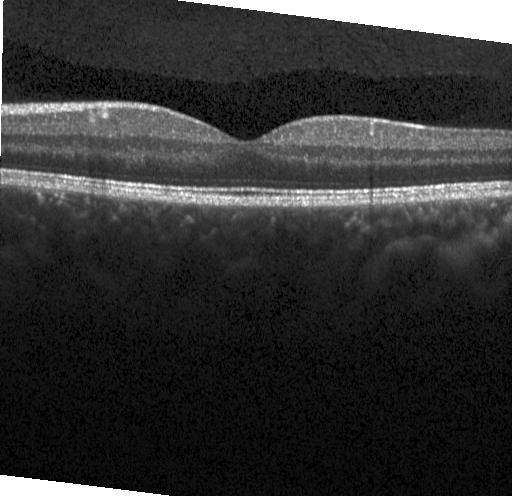

Through the macula; OCT line scan; spectral-domain optical coherence tomography; Heidelberg Spectralis. Assessment: no CNV, no DME, and no drusen.